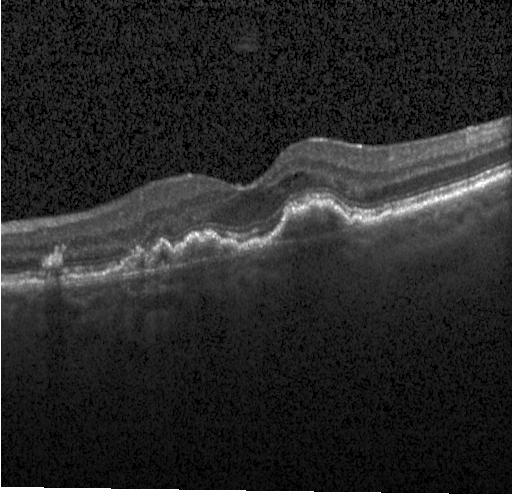
Optical coherence tomography scan. Spectral-domain OCT. Acquired on a Heidelberg Spectralis.
Diagnosis: choroidal neovascularization (CNV).